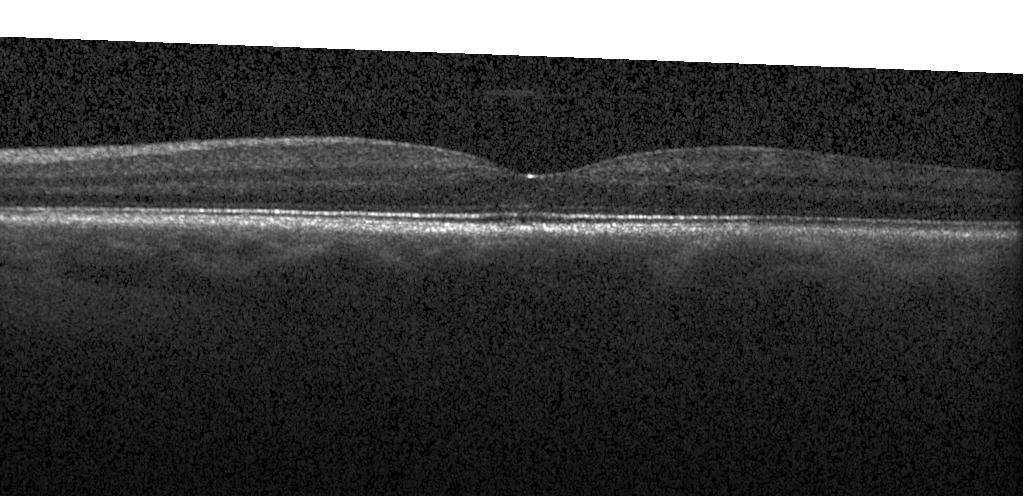

Acquired on a Heidelberg Spectralis; retinal OCT B-scan; SD-OCT — No CNV, DME, or drusen.